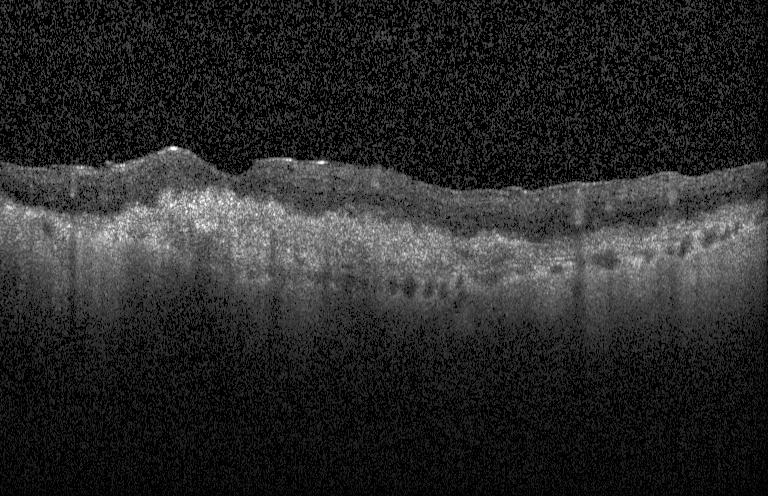 Finding: CNV.